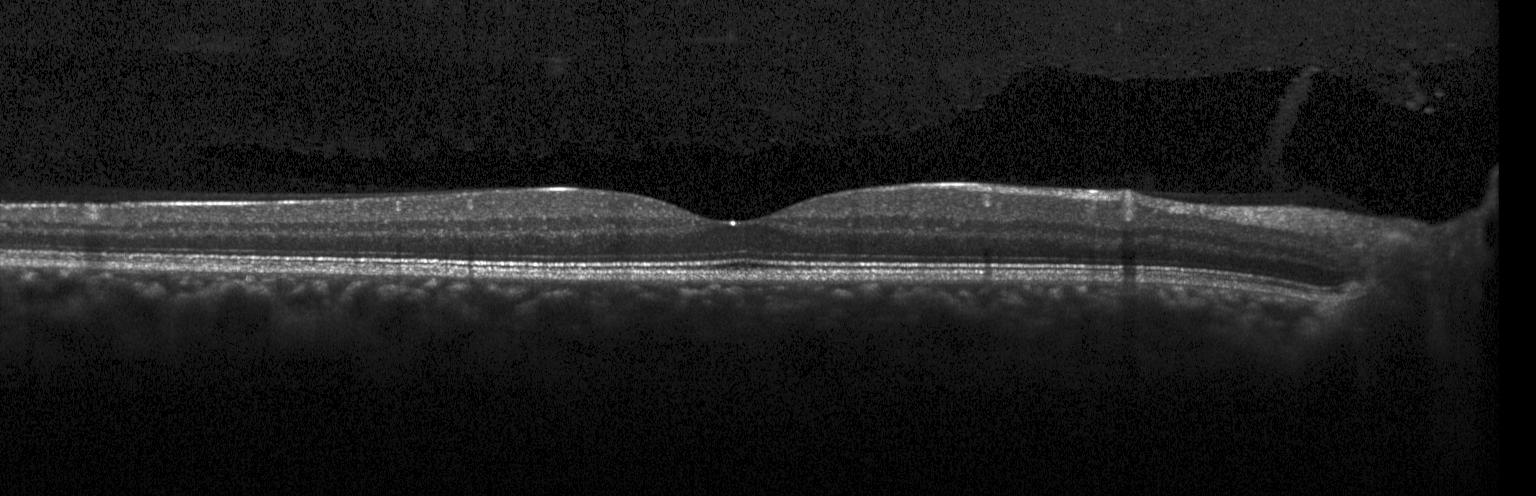

OCT line scan
The scan shows neither CNV, DME, nor drusen.